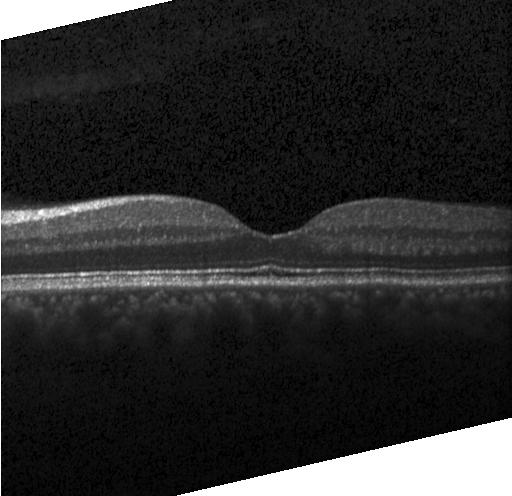
Spectral-domain OCT B-scan: no evidence of CNV, DME, or drusen.